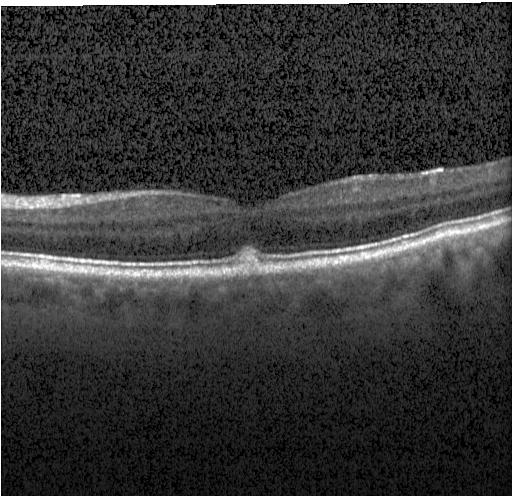

OCT B-scan. Assessment: drusen.